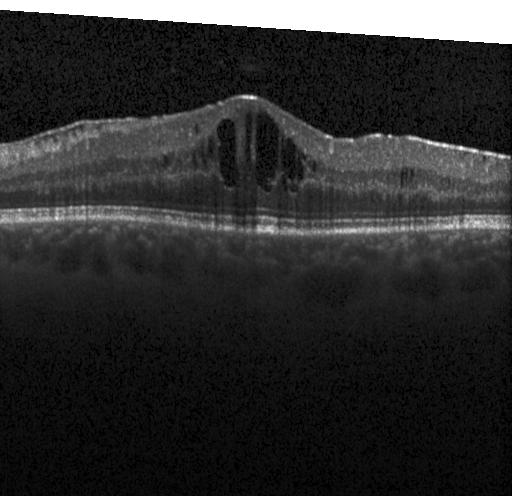
Optical coherence tomography B-scan; fovea-centered — Finding: diabetic macular edema.